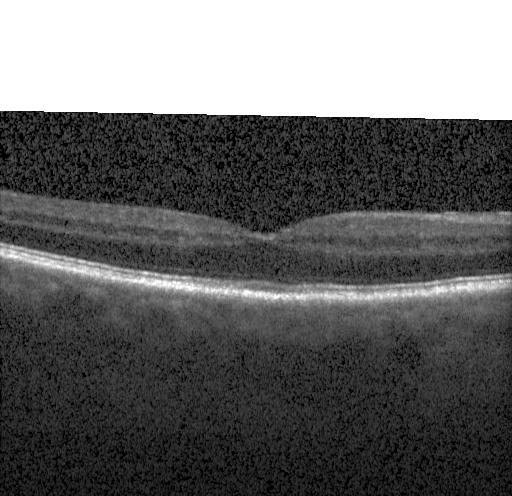

Horizontal scan through the fovea · Heidelberg Spectralis · optical coherence tomography scan
Diagnosis: no choroidal neovascularization, no diabetic macular edema, and no drusen.